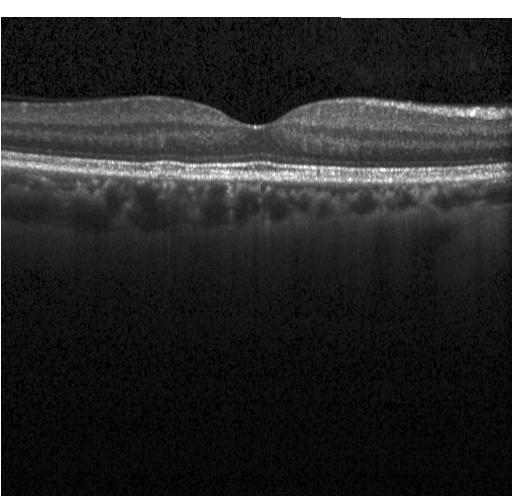 Spectral-domain OCT, fovea-centered, retinal OCT B-scan, Heidelberg Spectralis OCT system — This B-scan demonstrates multiple drusen.